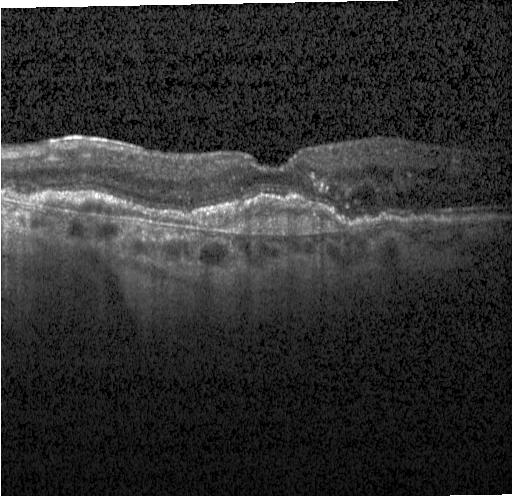
SD-OCT; macular scan; Heidelberg Spectralis; optical coherence tomography B-scan — Macular OCT: a choroidal neovascular membrane.